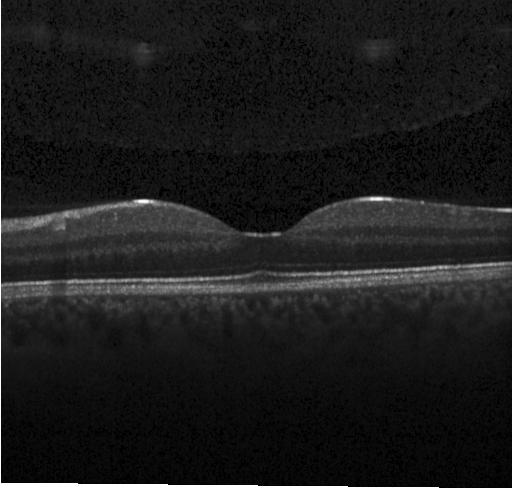 Spectral-domain OCT B-scan: no choroidal neovascularization, no diabetic macular edema, and no drusen.